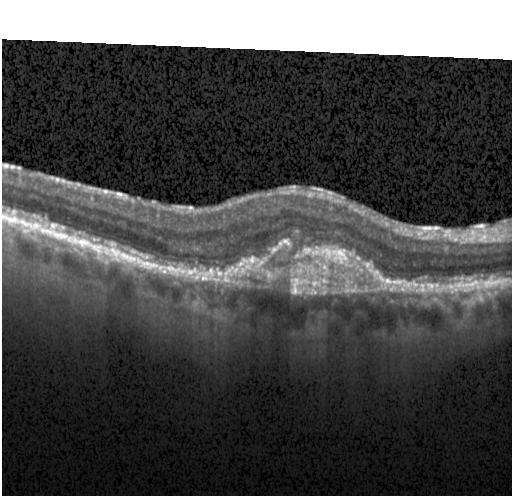 OCT scan showing a choroidal neovascular membrane.